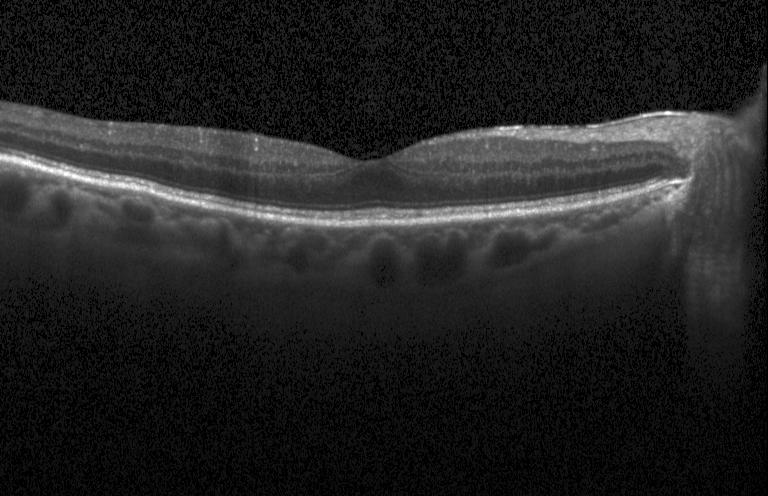

OCT line scan. This B-scan demonstrates no evidence of choroidal neovascularization, diabetic macular edema, or drusen.